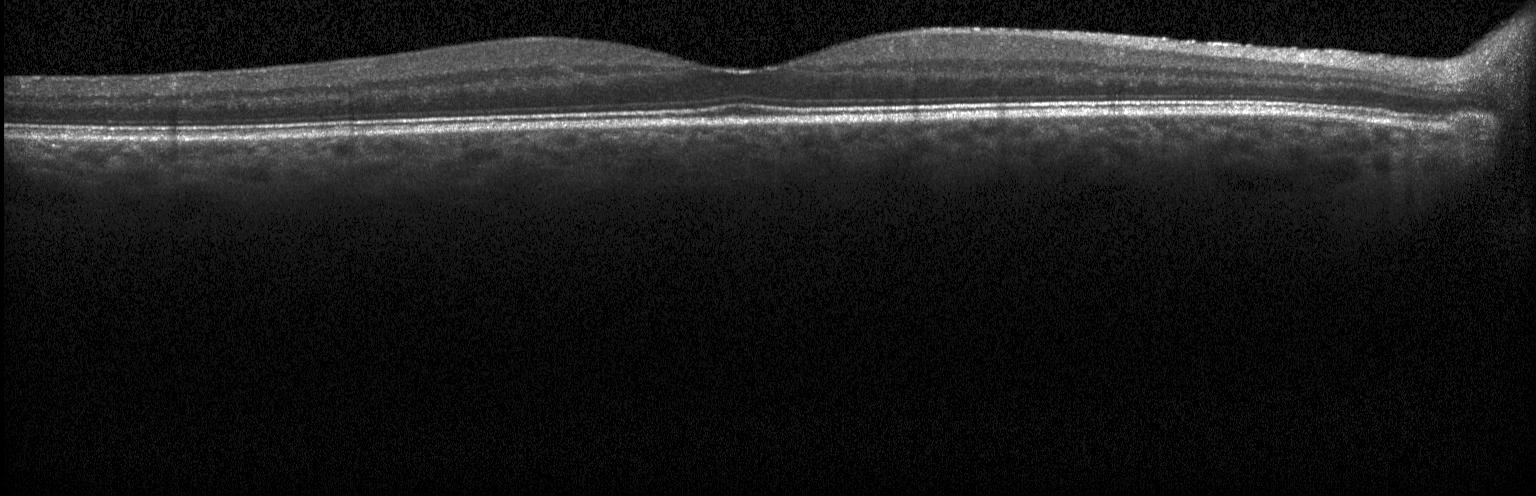 Finding: no choroidal neovascularization, diabetic macular edema, or drusen.